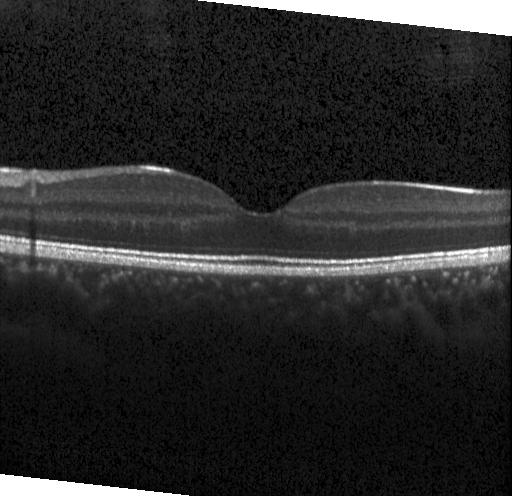

Macular OCT demonstrating neither CNV, DME, nor drusen.